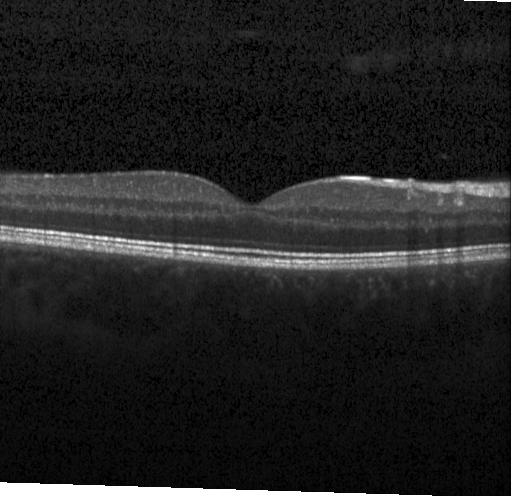

Spectral-domain OCT. Macular scan. Optical coherence tomography scan
Finding: no choroidal neovascularization, no diabetic macular edema, and no drusen.